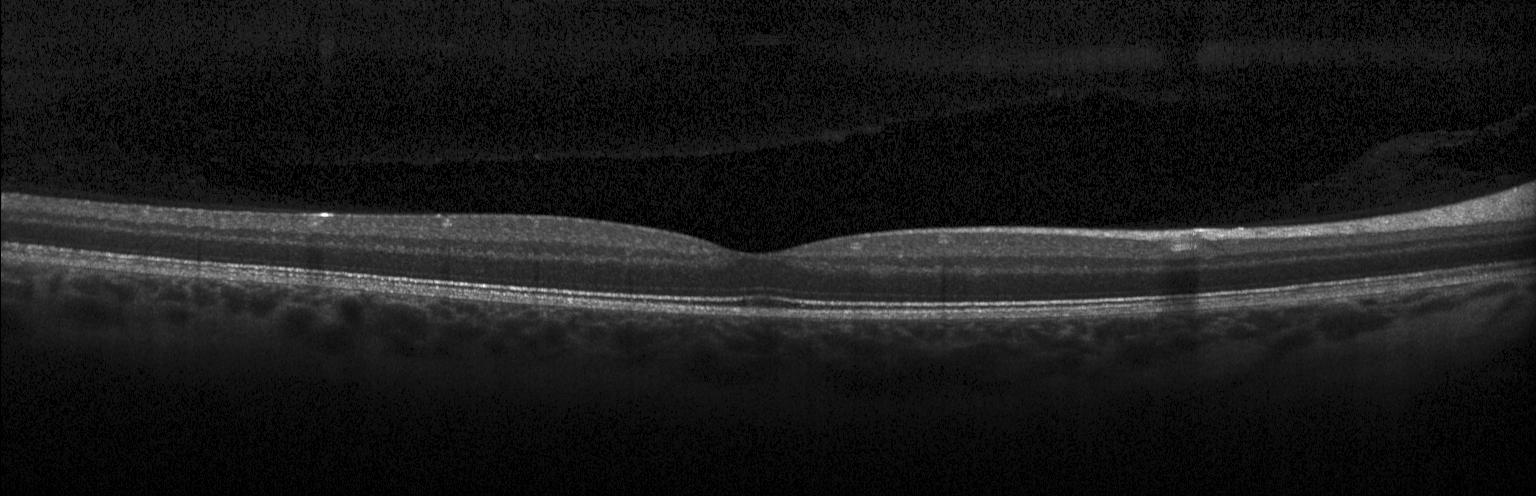
Diagnosis: neither CNV, DME, nor drusen.